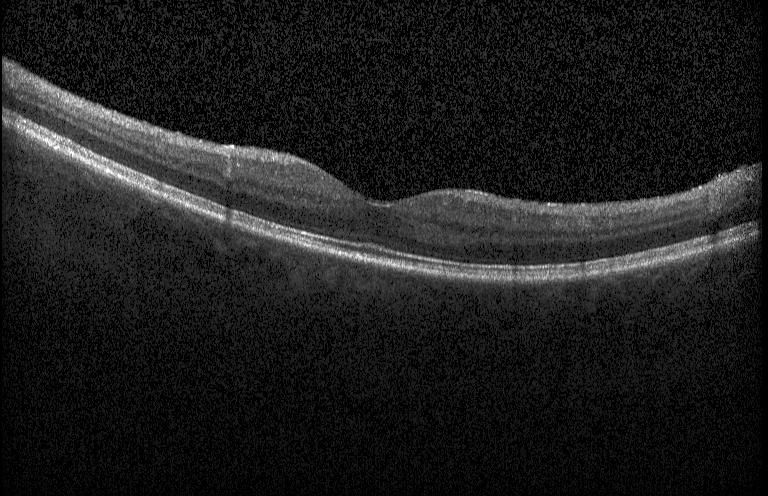

Impression: no choroidal neovascularization, diabetic macular edema, or drusen.